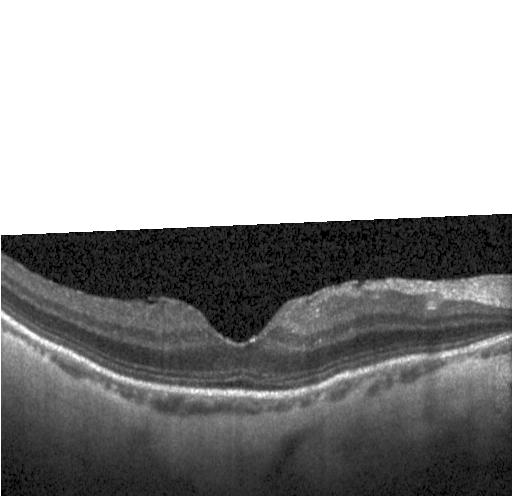 Macular OCT demonstrating no evidence of CNV, DME, or drusen.